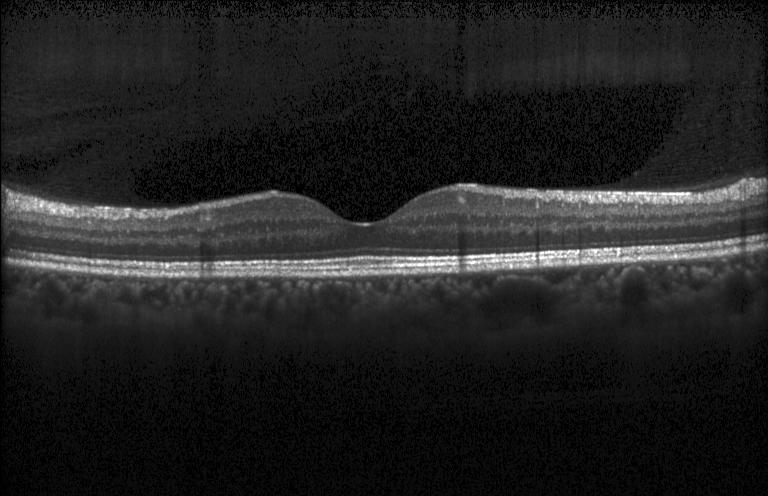 OCT finding: neither choroidal neovascularization, diabetic macular edema, nor drusen.